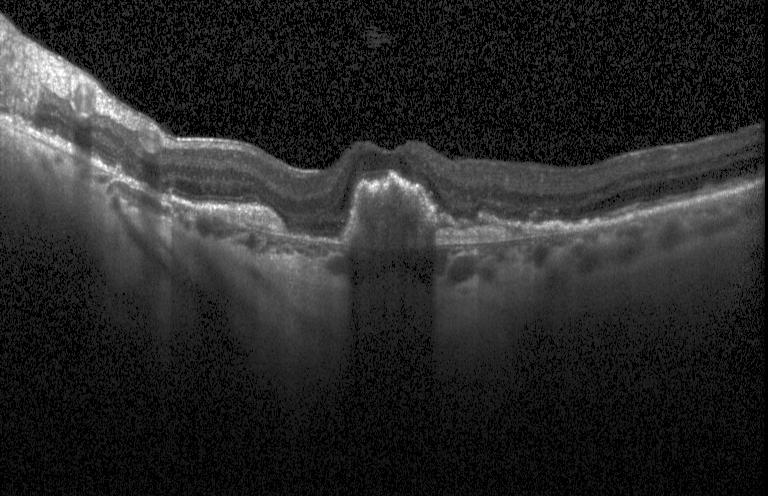

OCT line scan
Impression: choroidal neovascularization (CNV).